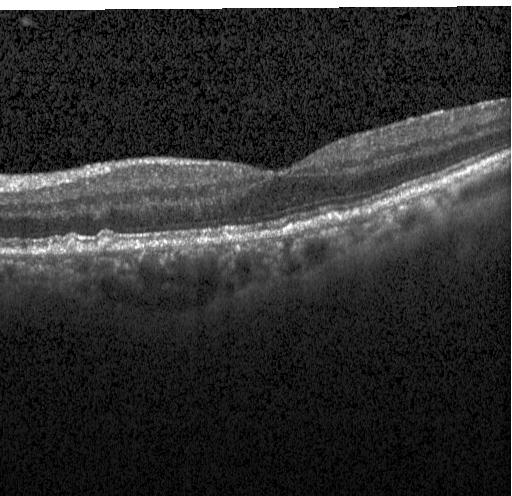

Assessment: drusen.